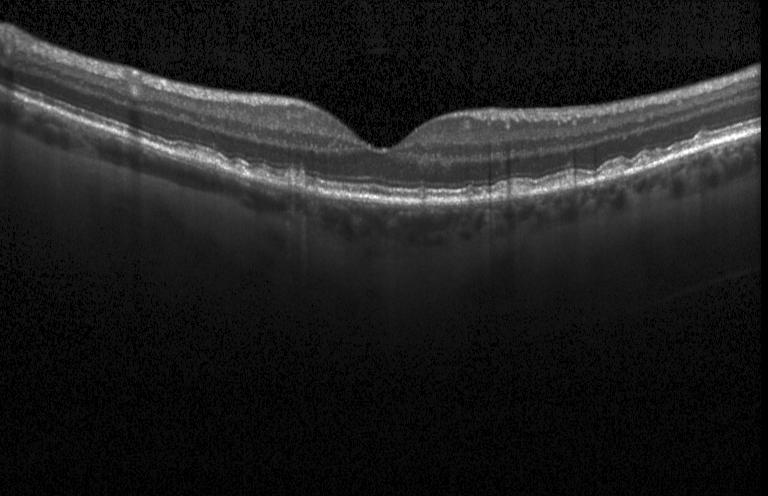
Spectral-domain optical coherence tomography, Heidelberg Spectralis OCT system, OCT line scan — Impression: drusen.